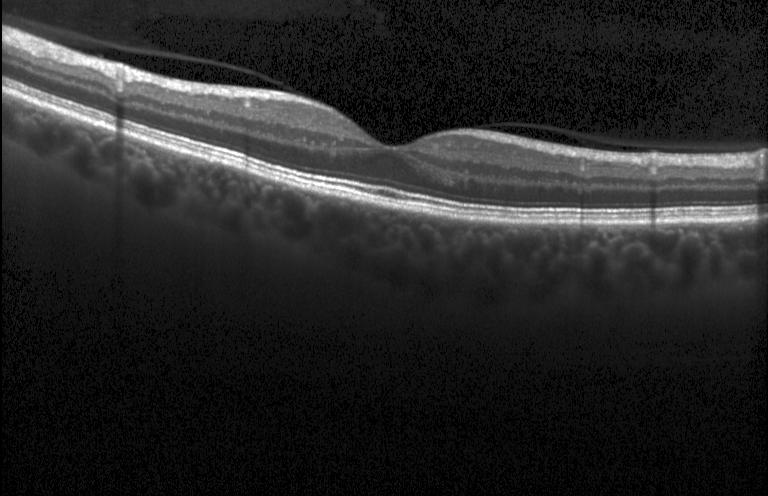
Finding: neither choroidal neovascularization, diabetic macular edema, nor drusen.